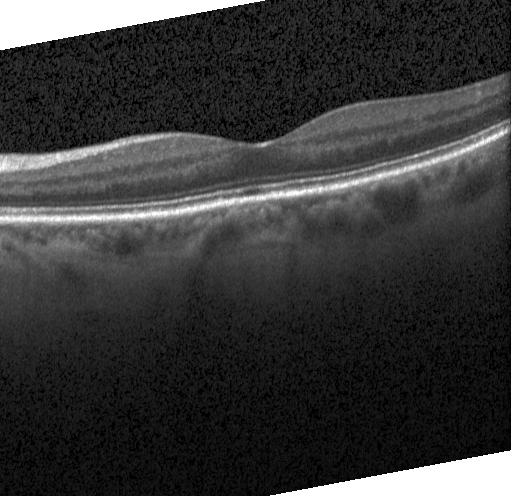
Finding: neither CNV, DME, nor drusen.